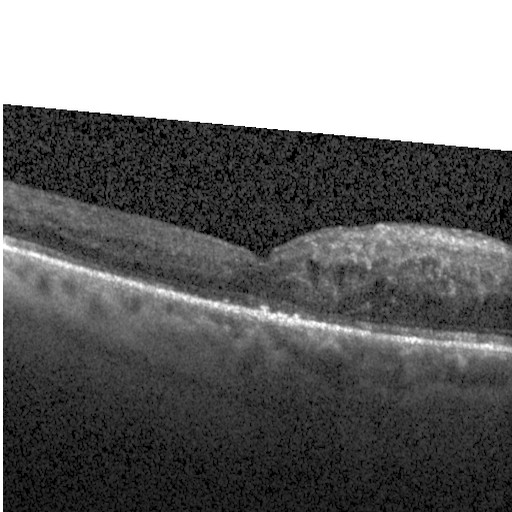
OCT finding: diabetic macular edema (DME).